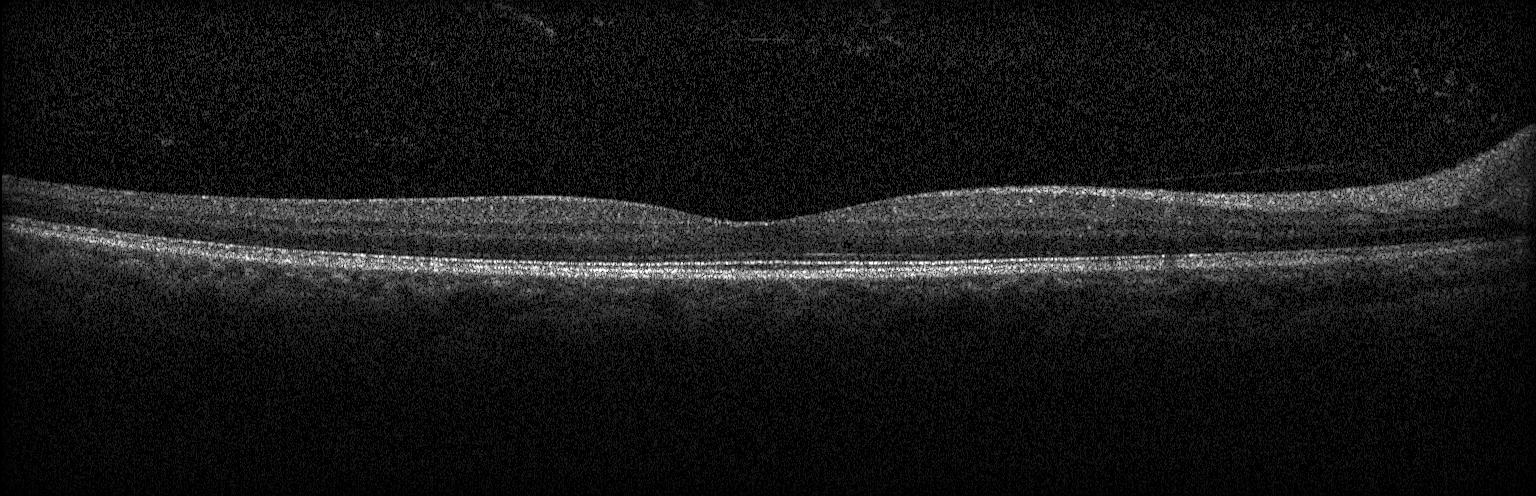 Retinal OCT B-scan. Diagnosis: no choroidal neovascularization, no diabetic macular edema, and no drusen.